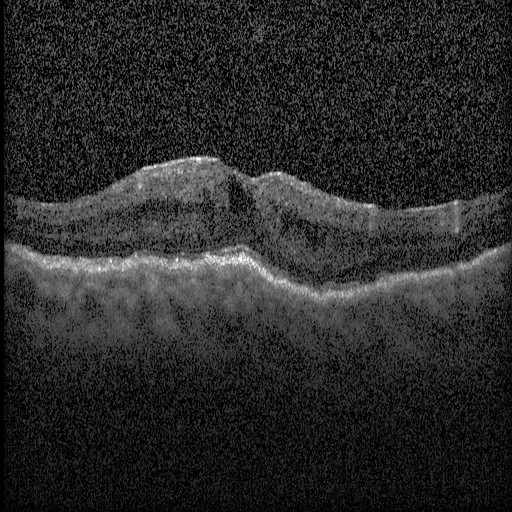 Optical coherence tomography B-scan. Dx: diabetic macular edema (DME).